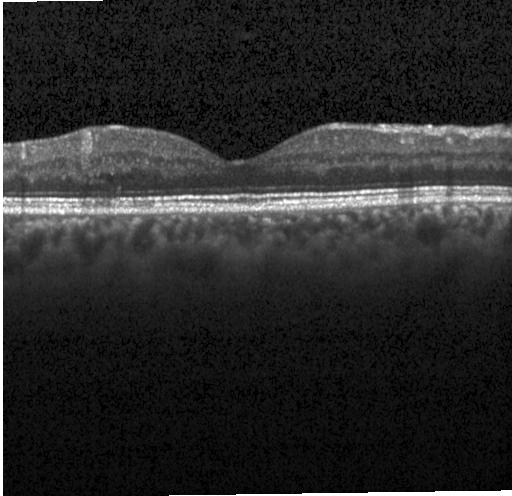

Horizontal scan through the fovea; optical coherence tomography B-scan.
Diagnosis: diabetic macular edema (DME).